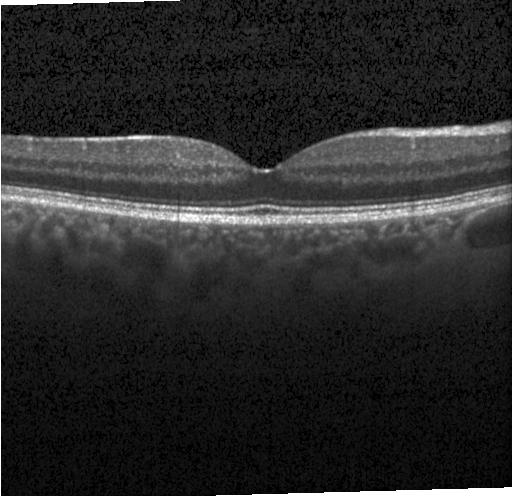
OCT scan showing no choroidal neovascularization, diabetic macular edema, or drusen.